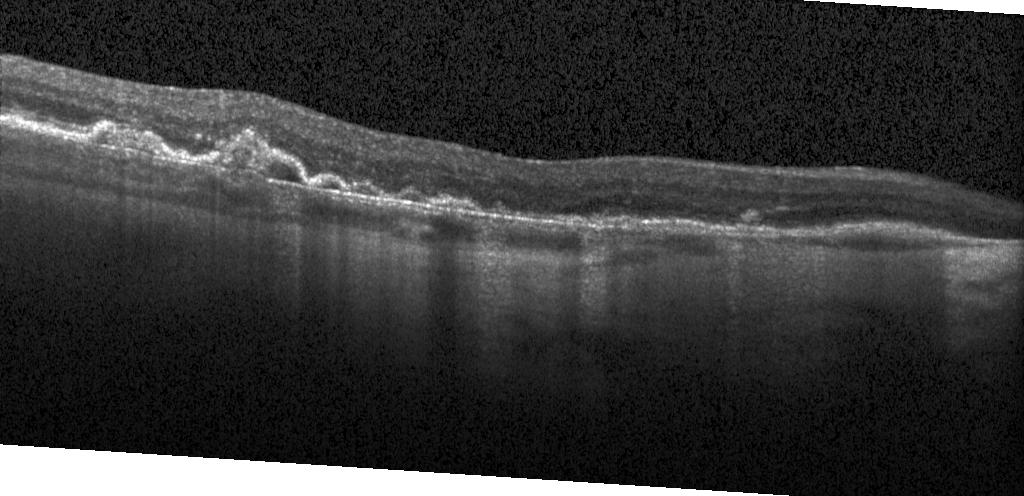
Retinal OCT B-scan · acquired on a Heidelberg Spectralis — Diagnosis: choroidal neovascularization.